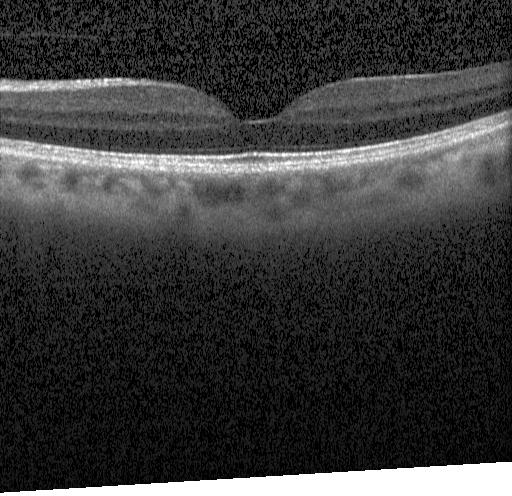 Retinal OCT cross-section
Diagnosis: no choroidal neovascularization, diabetic macular edema, or drusen.